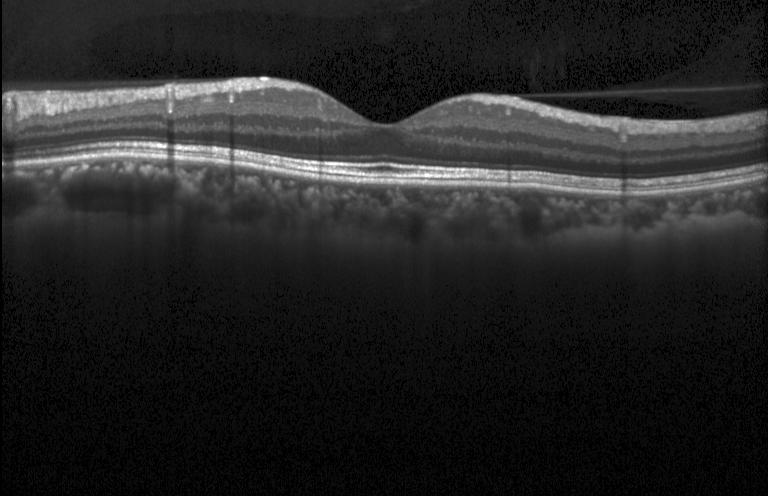 Instrument: Heidelberg Spectralis, spectral-domain optical coherence tomography, optical coherence tomography B-scan, fovea-centered. OCT finding: no CNV, no DME, and no drusen.